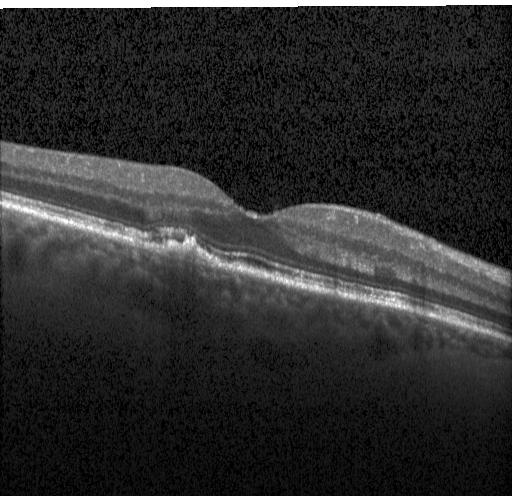

Heidelberg Spectralis. Centered on the fovea. Optical coherence tomography scan. SD-OCT.
The scan shows choroidal neovascularization (CNV).